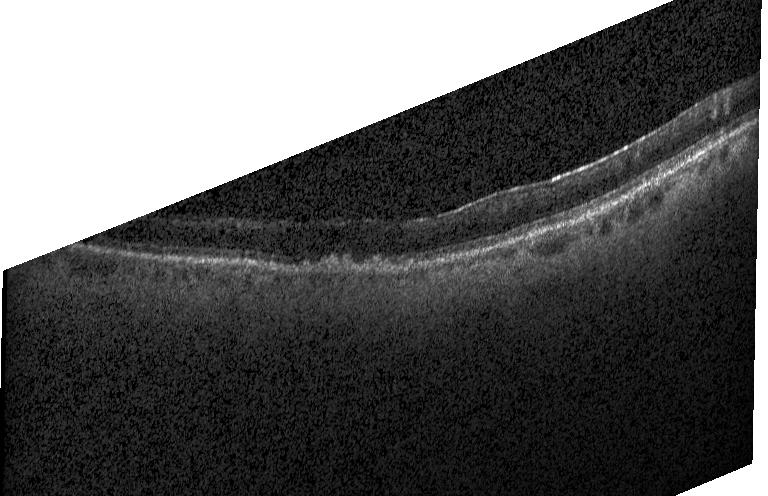

Heidelberg Spectralis OCT system. Retinal OCT cross-section. Through the macula
This B-scan demonstrates sub-RPE drusenoid deposits.